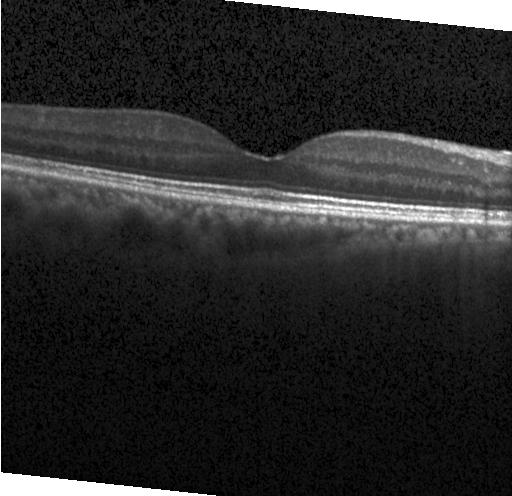 Through the macula · optical coherence tomography scan
Impression: no CNV, no DME, and no drusen.